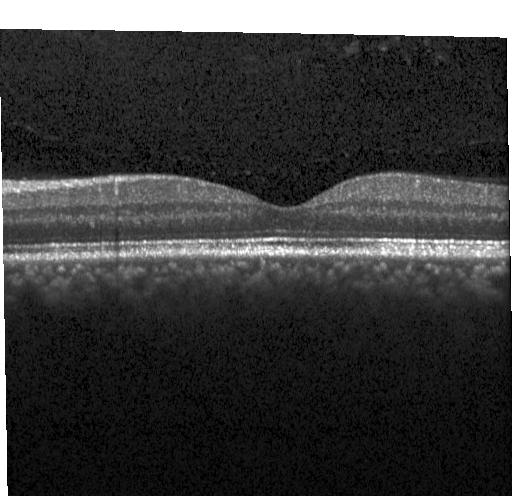 Optical coherence tomography scan · acquired on a Heidelberg Spectralis.
Neither choroidal neovascularization, diabetic macular edema, nor drusen.